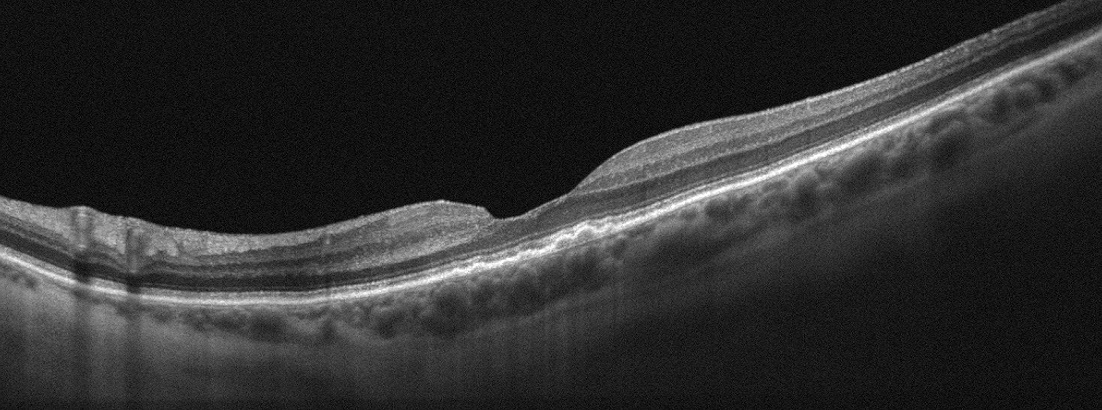 Through the macula · retinal OCT cross-section · Optovue Avanti RTVue XR — Diagnosis: AMD.